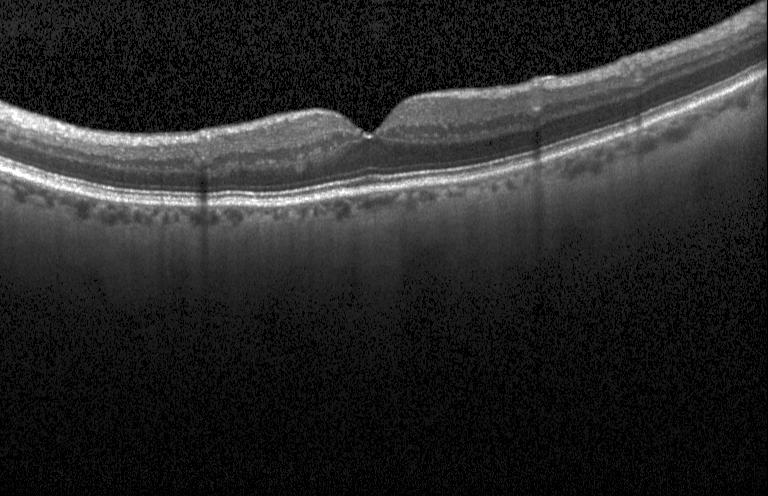

Heidelberg Spectralis; retinal OCT B-scan; spectral-domain OCT — The scan shows neither choroidal neovascularization, diabetic macular edema, nor drusen.